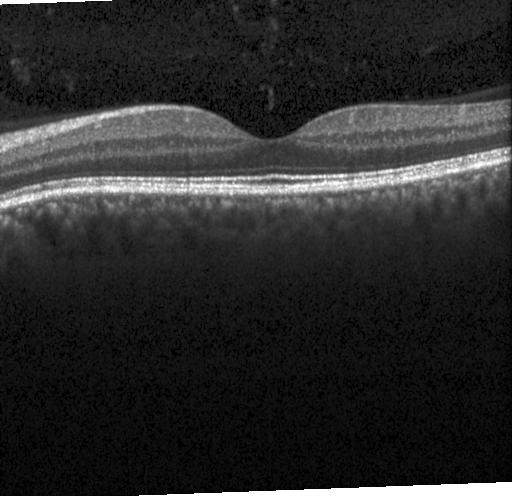 Heidelberg Spectralis OCT system; SD-OCT; optical coherence tomography scan; fovea-centered
No choroidal neovascularization, diabetic macular edema, or drusen.